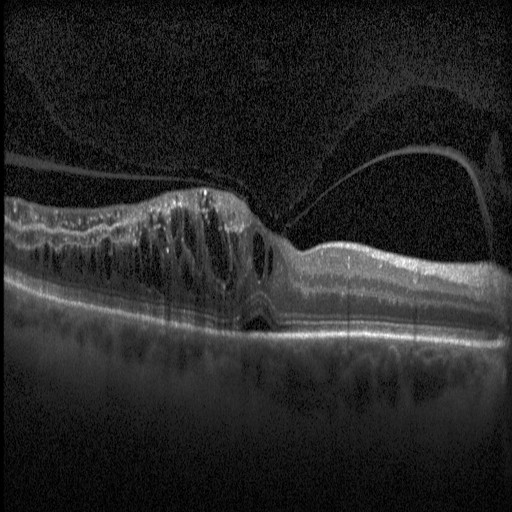

The scan shows diabetic macular edema (DME).